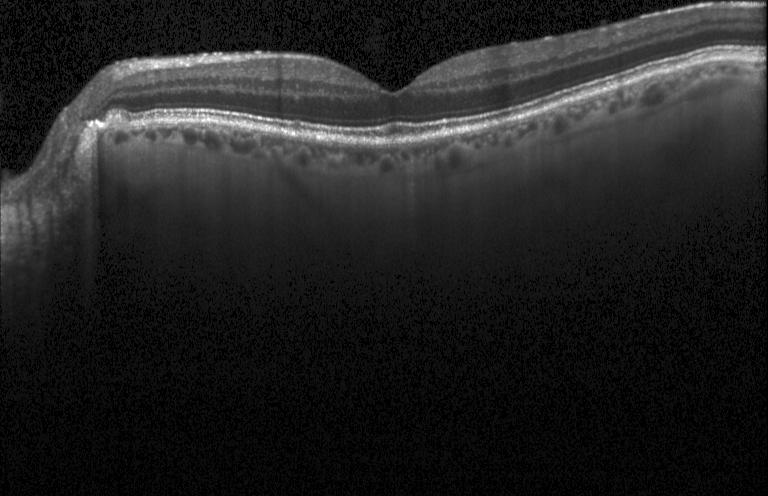 Dx: no evidence of CNV, DME, or drusen.